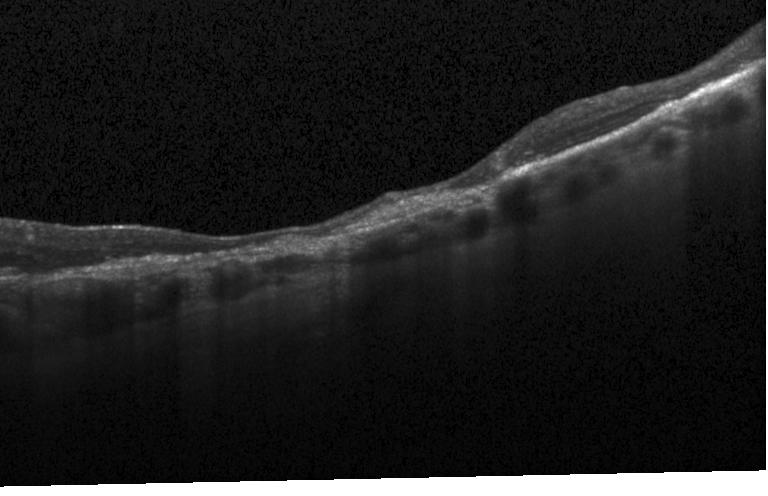 Retinal OCT B-scan
Impression: CNV.